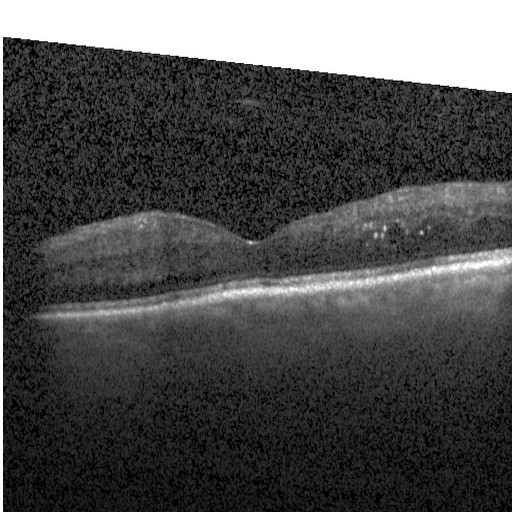
Diagnosis: DME.